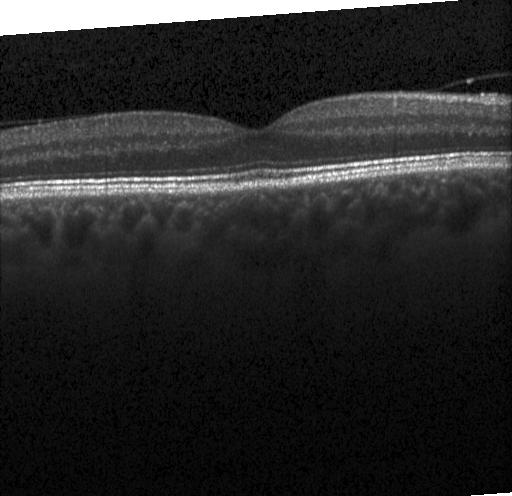
Retinal OCT cross-section. Heidelberg Spectralis. Through the macula. SD-OCT.
Diagnosis: no evidence of CNV, DME, or drusen.